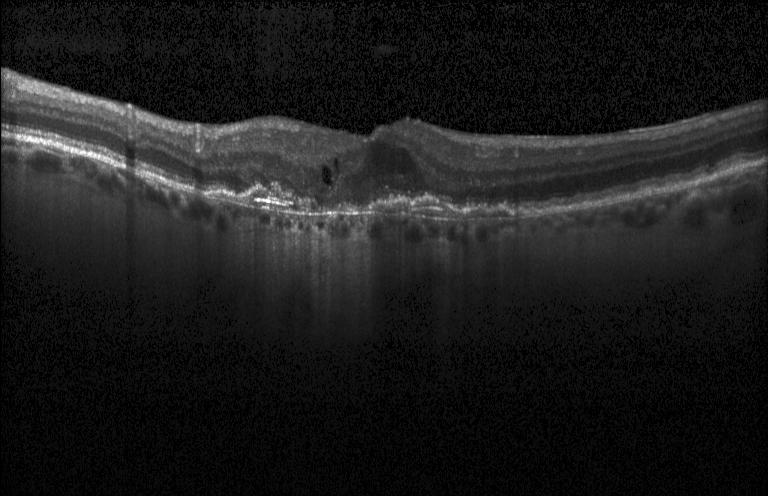

OCT line scan. Impression: choroidal neovascularization.